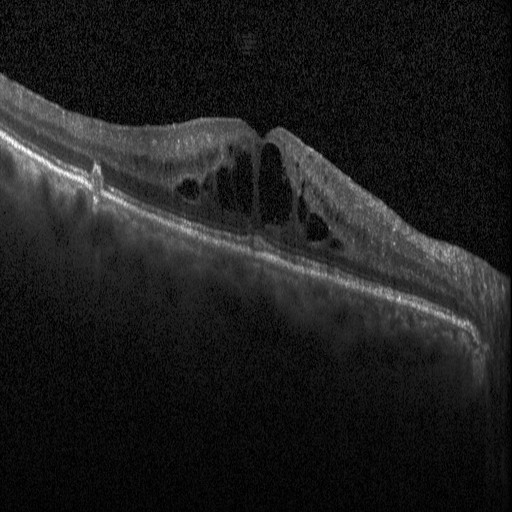 OCT B-scan, macular scan, spectral-domain optical coherence tomography, instrument: Heidelberg Spectralis. Macular OCT: DME.